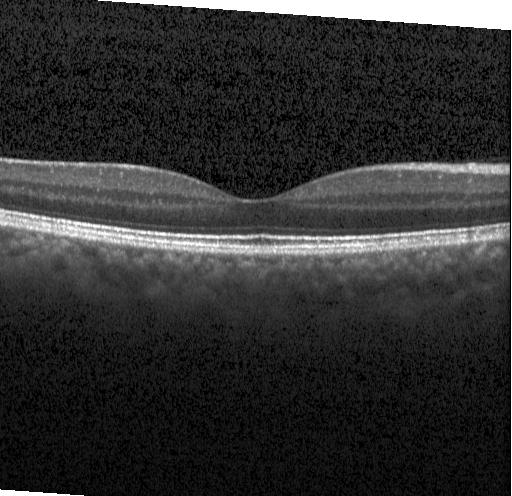
Dx: no choroidal neovascularization, diabetic macular edema, or drusen.